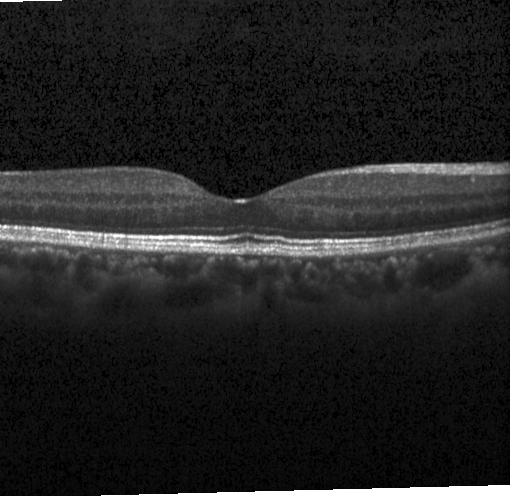
Finding: no evidence of CNV, DME, or drusen.